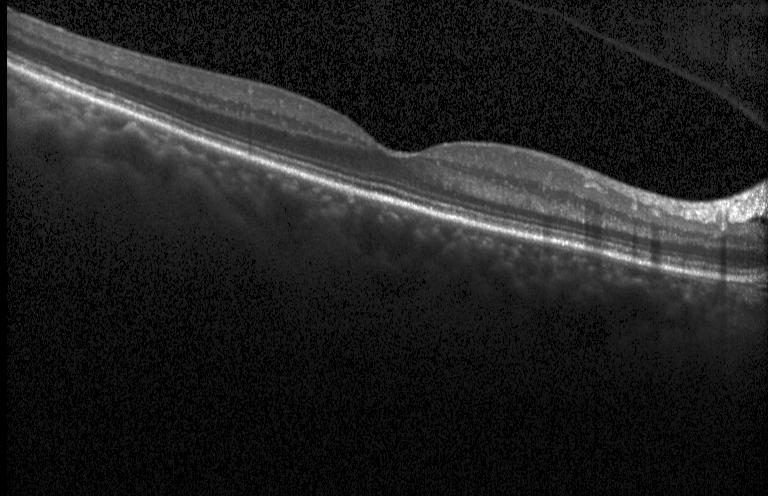

Finding: no choroidal neovascularization, no diabetic macular edema, and no drusen.